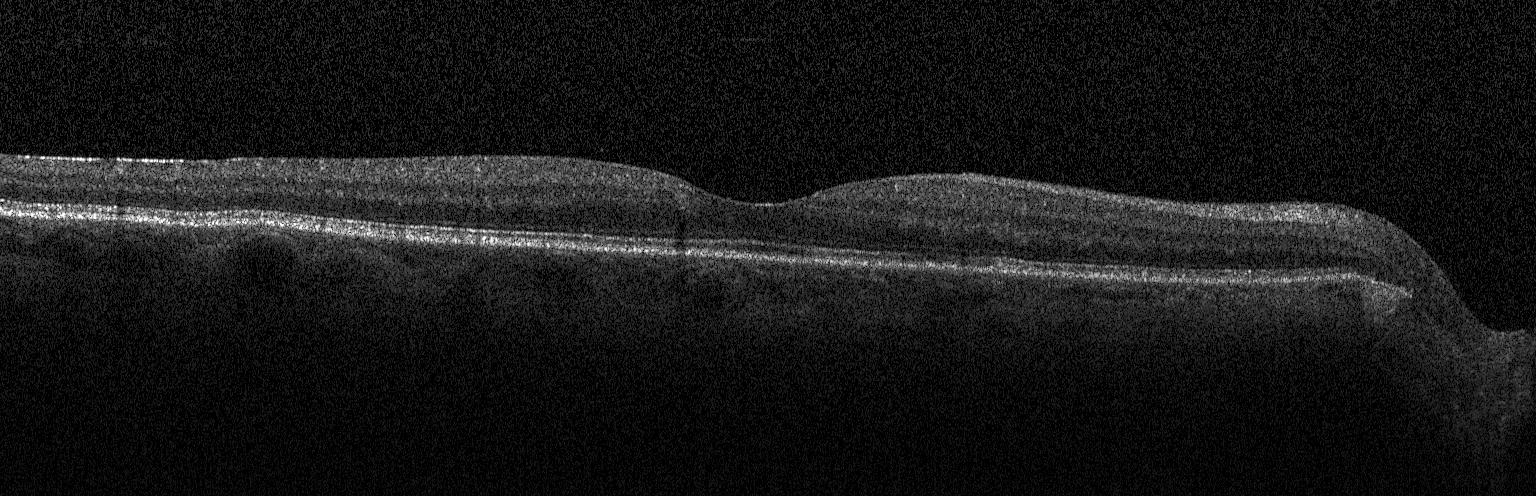
Finding: neither choroidal neovascularization, diabetic macular edema, nor drusen.